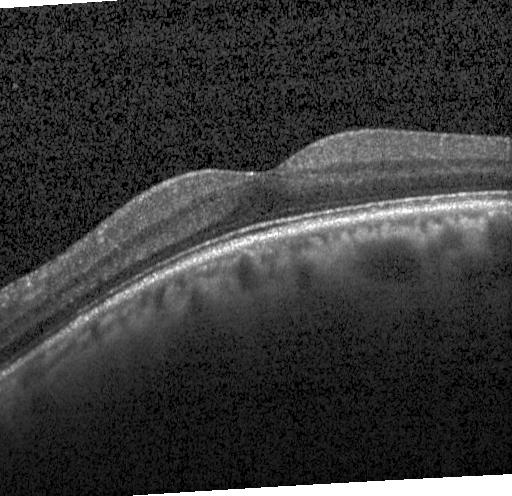 Macular OCT demonstrating no CNV, no DME, and no drusen.